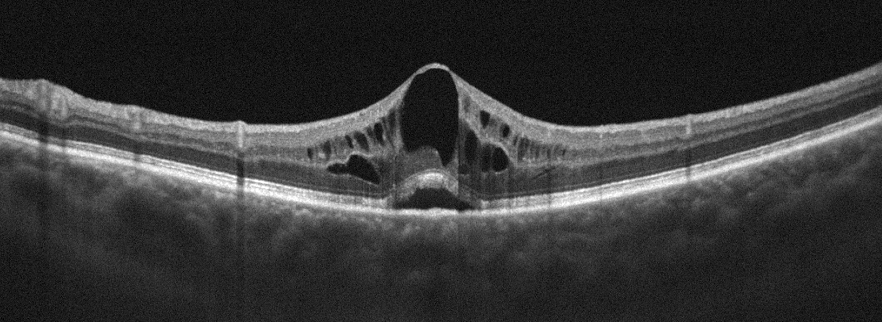 OS · OCT B-scan.
The scan shows retinal vein occlusion (RVO).